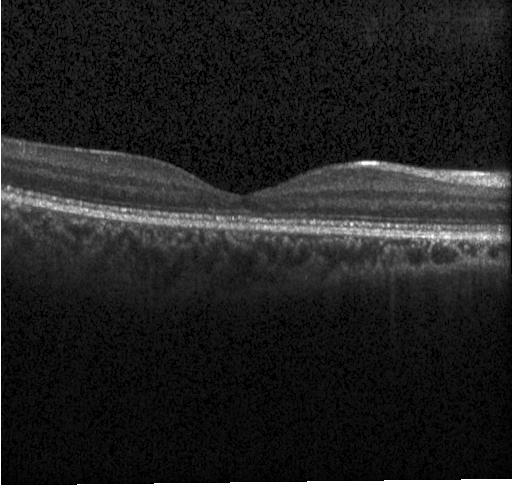
OCT line scan
The scan shows neither choroidal neovascularization, diabetic macular edema, nor drusen.